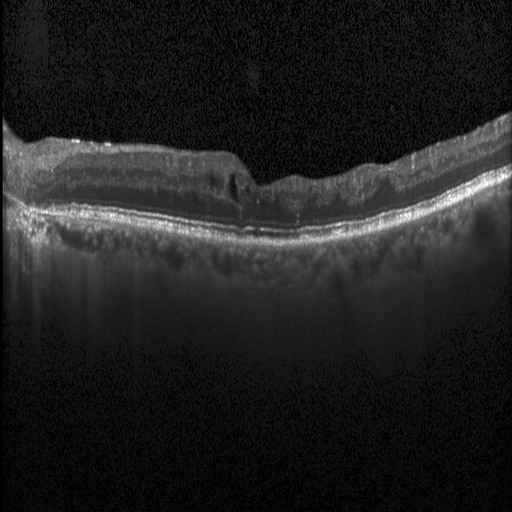

Optical coherence tomography B-scan. Heidelberg Spectralis
Diagnosis: DME.